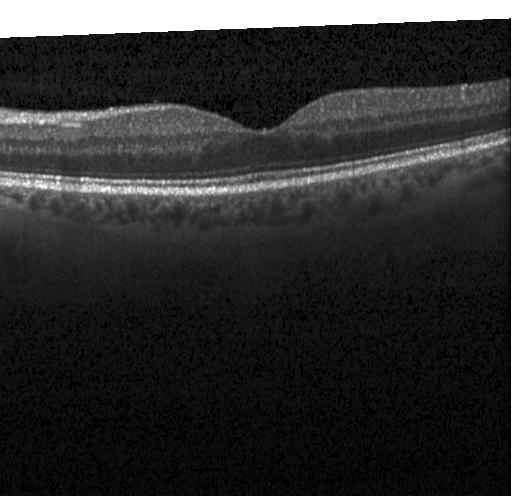
OCT line scan; spectral-domain optical coherence tomography.
Impression: no choroidal neovascularization, diabetic macular edema, or drusen.